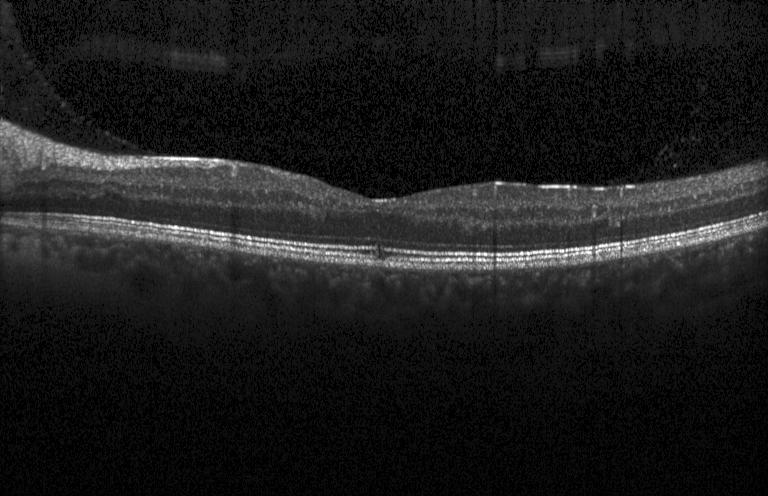

Spectral-domain OCT · optical coherence tomography scan.
Diagnosis: neither choroidal neovascularization, diabetic macular edema, nor drusen.